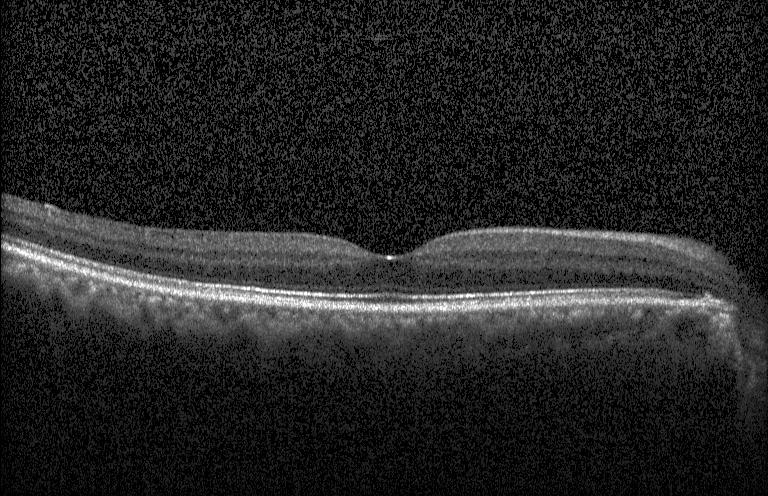

OCT B-scan showing neither choroidal neovascularization, diabetic macular edema, nor drusen.